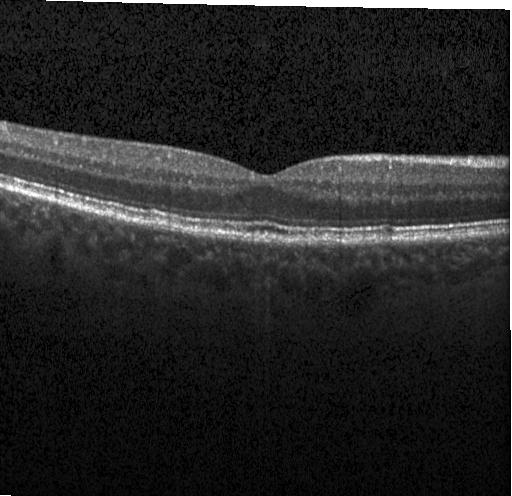

Spectral-domain optical coherence tomography; horizontal scan through the fovea; optical coherence tomography B-scan; instrument: Heidelberg Spectralis — Dx: drusen.